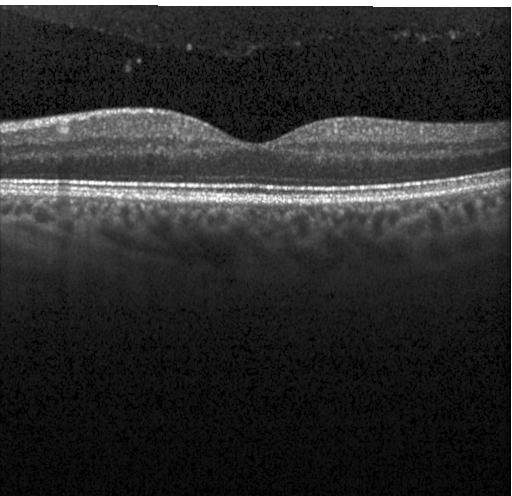 OCT line scan, through the macula, spectral-domain optical coherence tomography
Finding: no CNV, no DME, and no drusen.